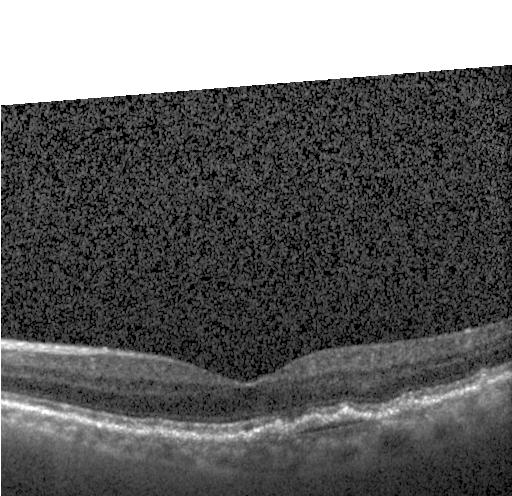
This B-scan demonstrates a choroidal neovascular membrane.